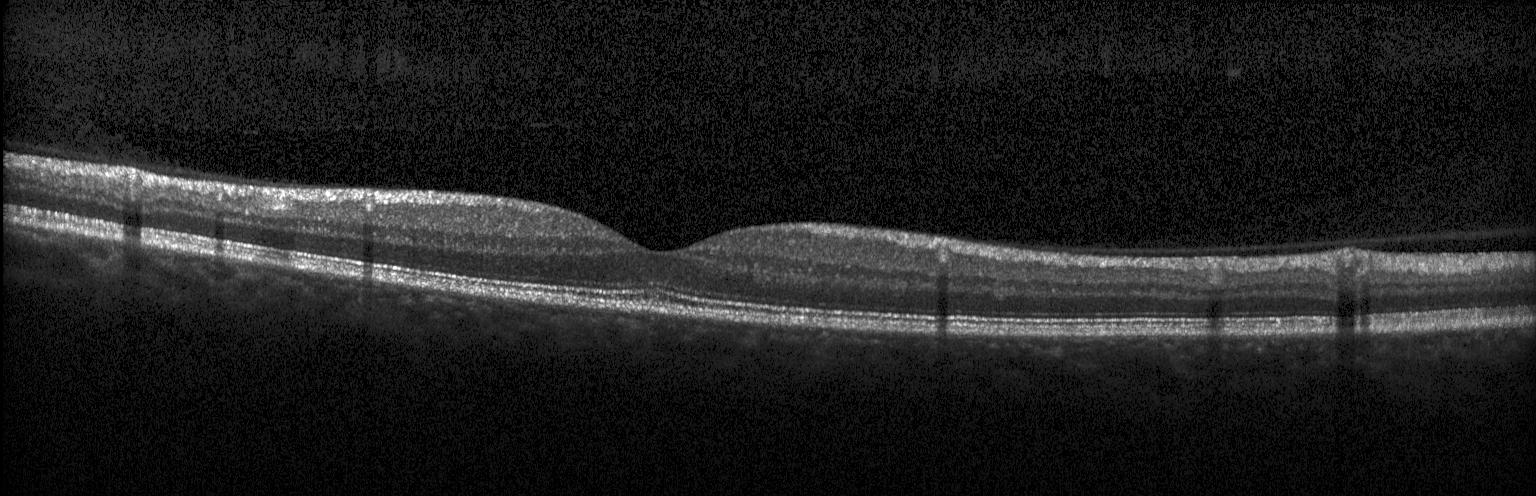

Optical coherence tomography scan. Heidelberg Spectralis OCT system — Macular OCT: neither choroidal neovascularization, diabetic macular edema, nor drusen.